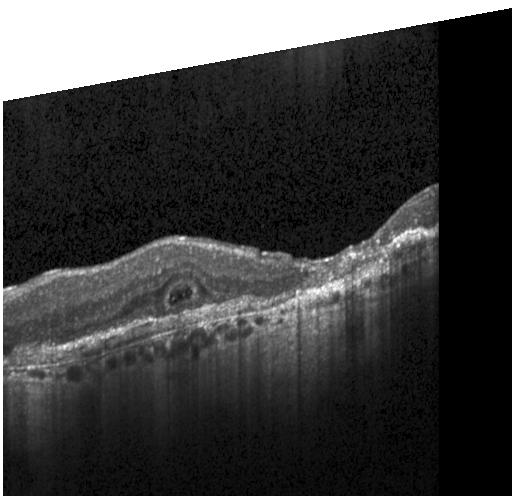

Retinal OCT cross-section. Instrument: Heidelberg Spectralis. Fovea-centered. Spectral-domain OCT. Impression: CNV.